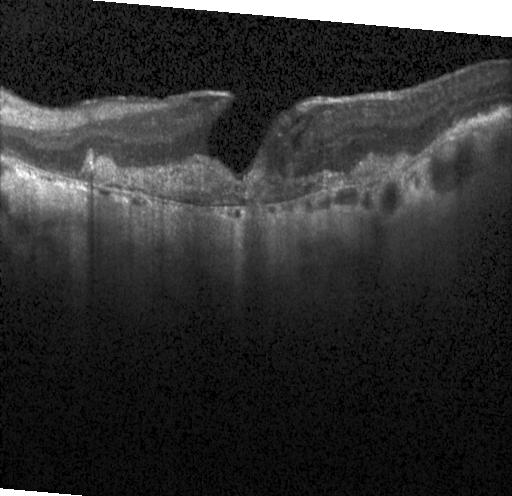
Optical coherence tomography scan
Impression: a choroidal neovascular membrane.